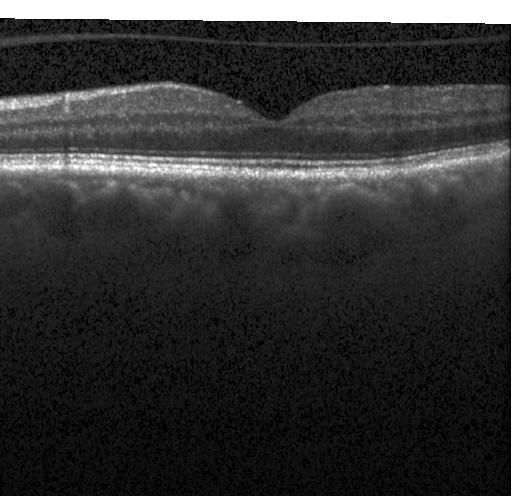 Retinal OCT cross-section. Heidelberg Spectralis.
The scan shows no CNV, no DME, and no drusen.